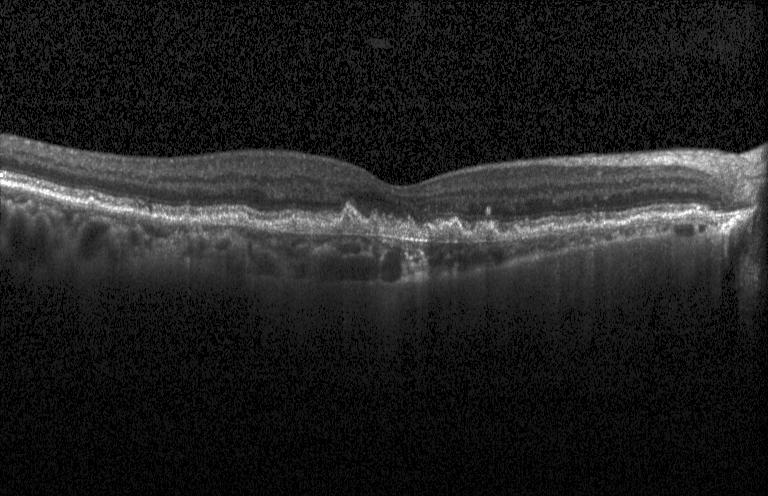 Dx: CNV.